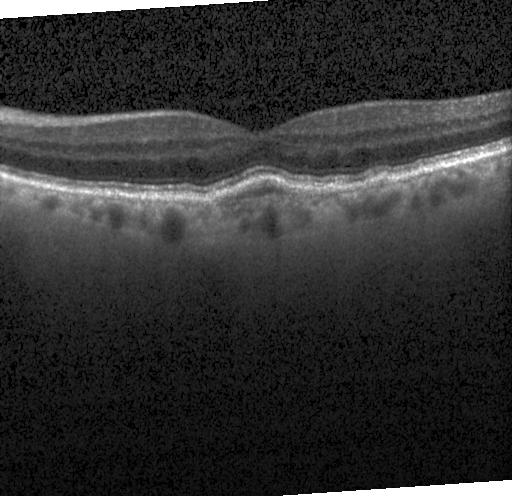

Spectral-domain OCT B-scan: choroidal neovascularization (CNV).